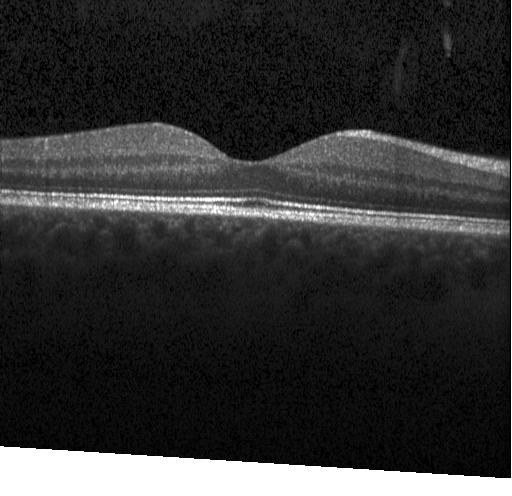 OCT B-scan · Heidelberg Spectralis OCT system · horizontal scan through the fovea · SD-OCT. Diagnosis: neither choroidal neovascularization, diabetic macular edema, nor drusen.